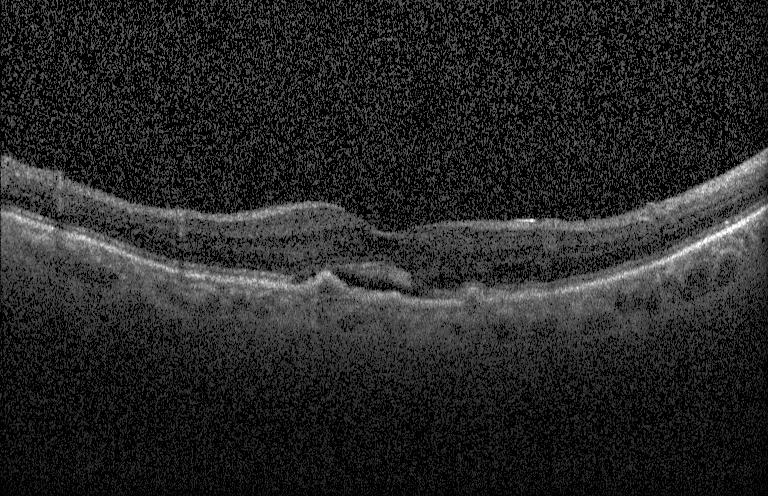 Spectral-domain OCT B-scan: a choroidal neovascular membrane.